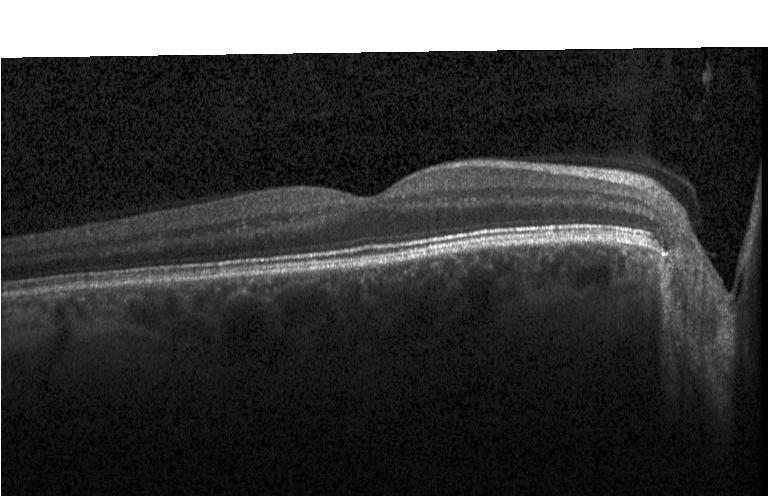 Impression: no CNV, no DME, and no drusen.